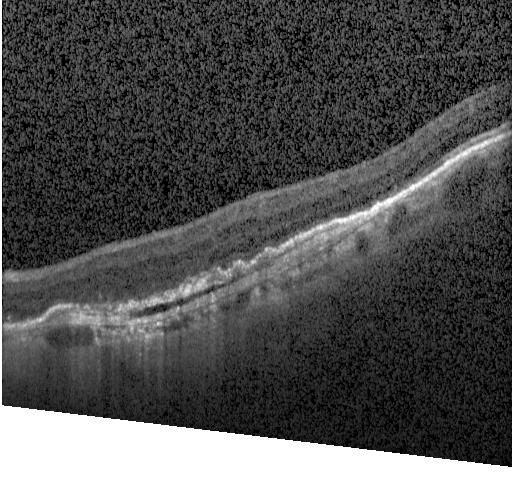

Diagnosis: a choroidal neovascular membrane.